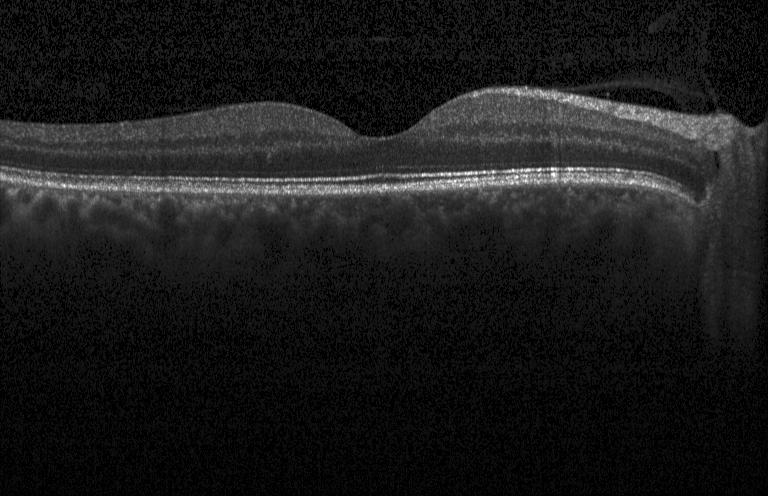 Retinal OCT cross-section
Dx: no evidence of CNV, DME, or drusen.